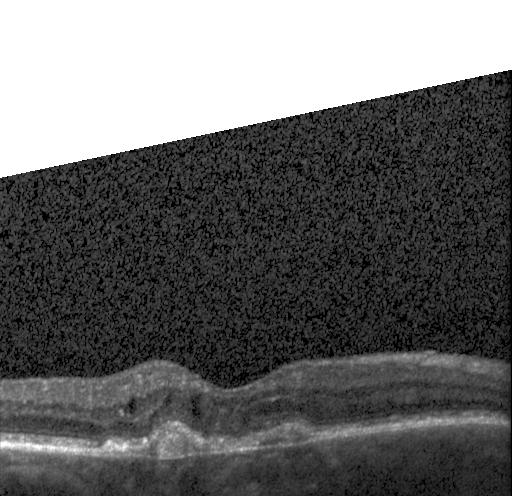
Diagnosis: CNV.